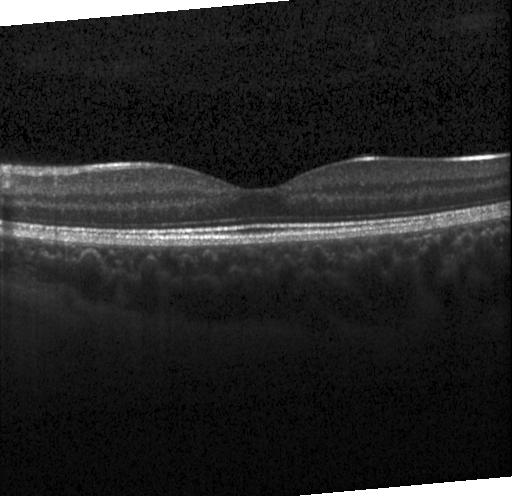
Assessment: no CNV, DME, or drusen.